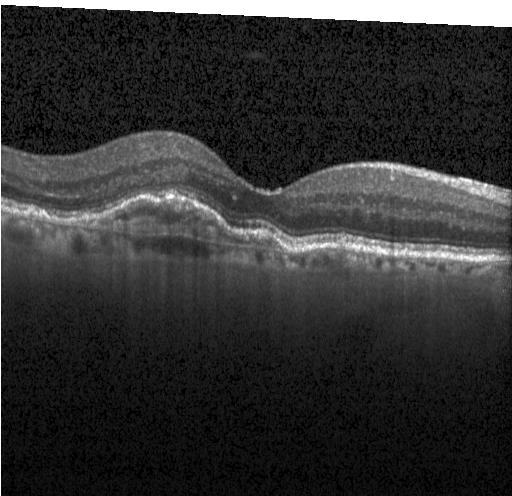

CNV.